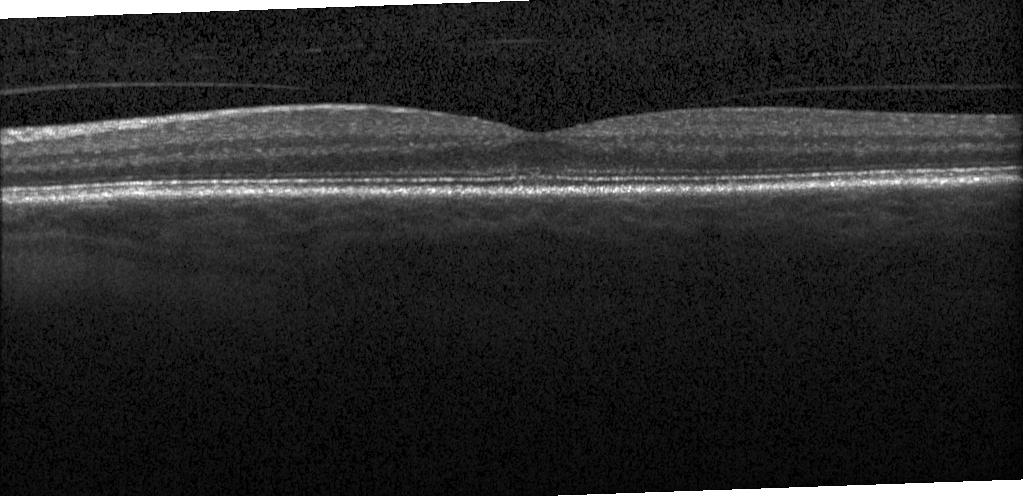
This B-scan demonstrates neither choroidal neovascularization, diabetic macular edema, nor drusen.